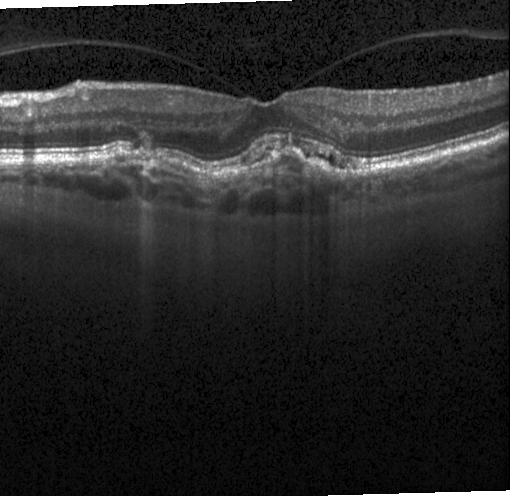
Retinal OCT cross-section; spectral-domain optical coherence tomography — Assessment: a choroidal neovascular membrane.